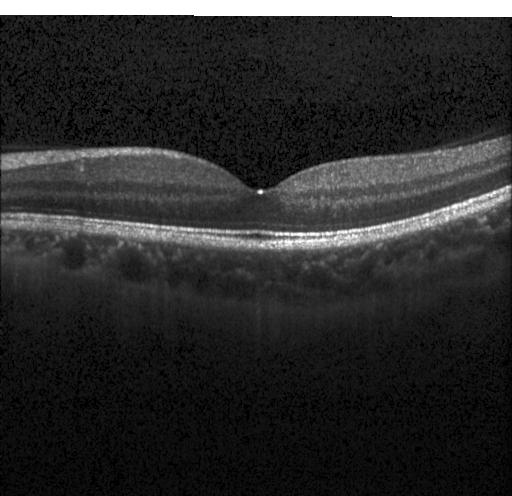
Through the macula. Retinal OCT cross-section. SD-OCT
Finding: no choroidal neovascularization, diabetic macular edema, or drusen.